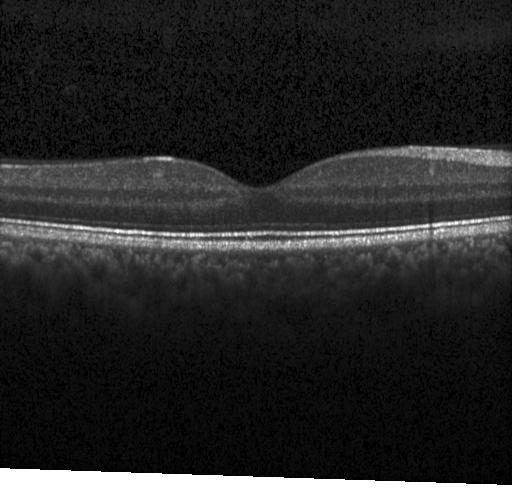

Horizontal scan through the fovea. Spectral-domain OCT. Optical coherence tomography B-scan
No evidence of choroidal neovascularization, diabetic macular edema, or drusen.